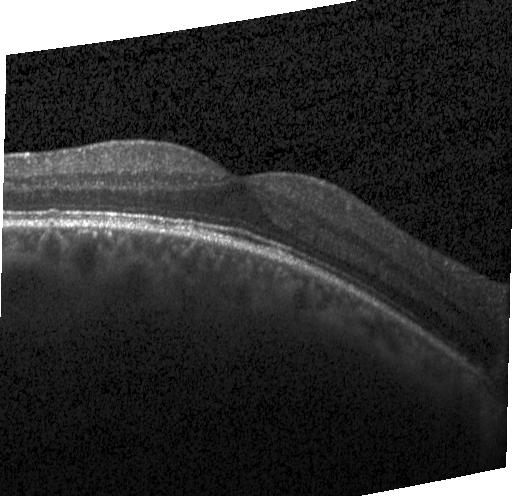
OCT scan showing no evidence of choroidal neovascularization, diabetic macular edema, or drusen.